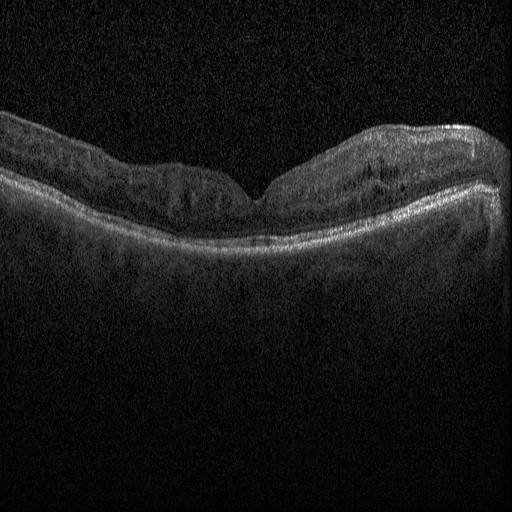

Spectral-domain OCT B-scan: diabetic macular edema (DME).